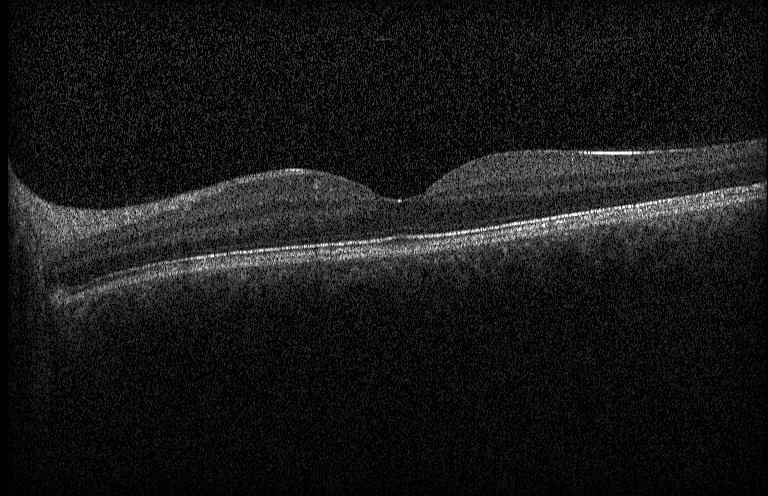

Finding: no evidence of choroidal neovascularization, diabetic macular edema, or drusen.